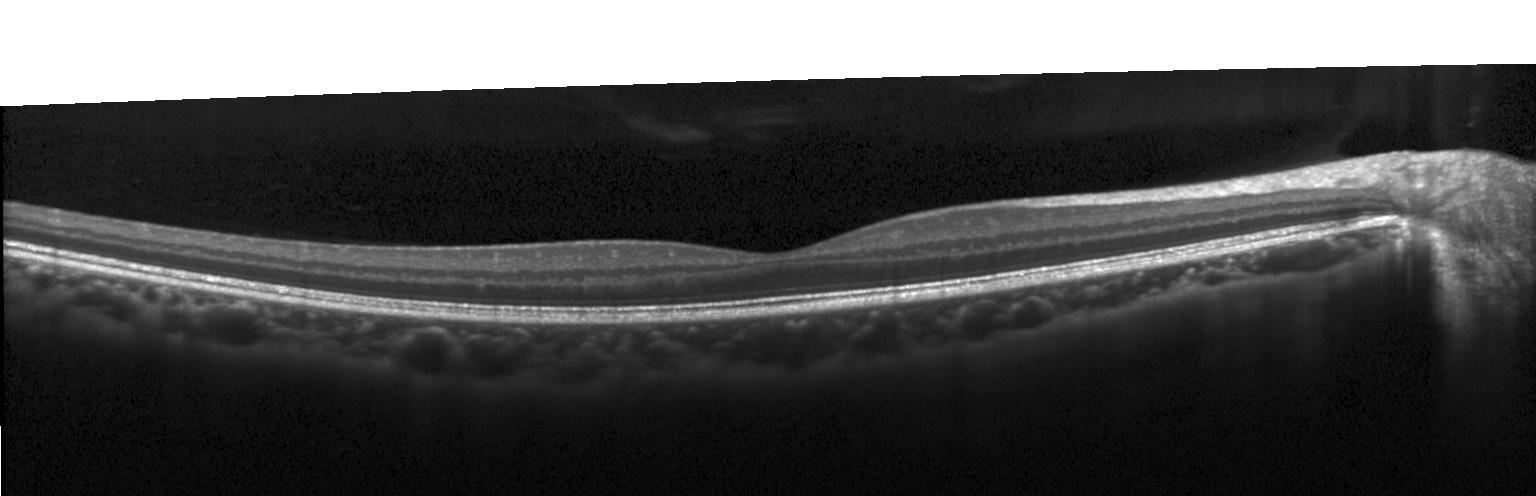
OCT line scan — The scan shows neither choroidal neovascularization, diabetic macular edema, nor drusen.